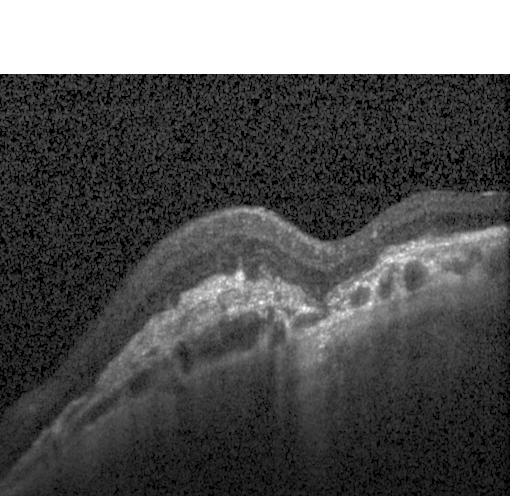 Impression: CNV.